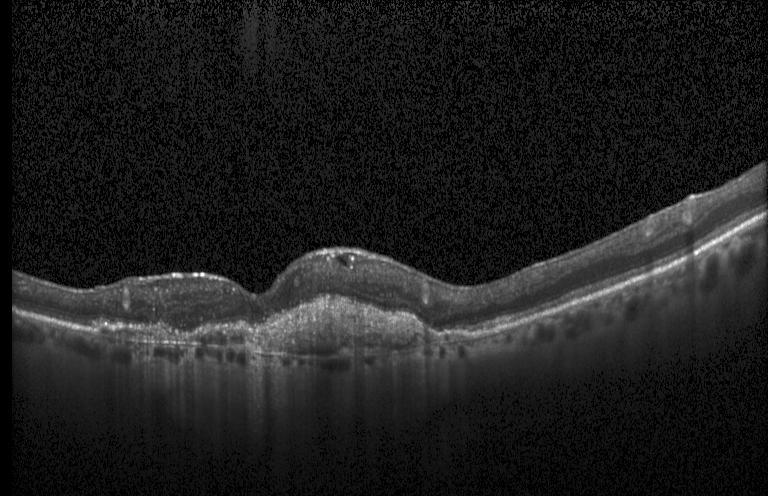 Optical coherence tomography B-scan — Diagnosis: a choroidal neovascular membrane.